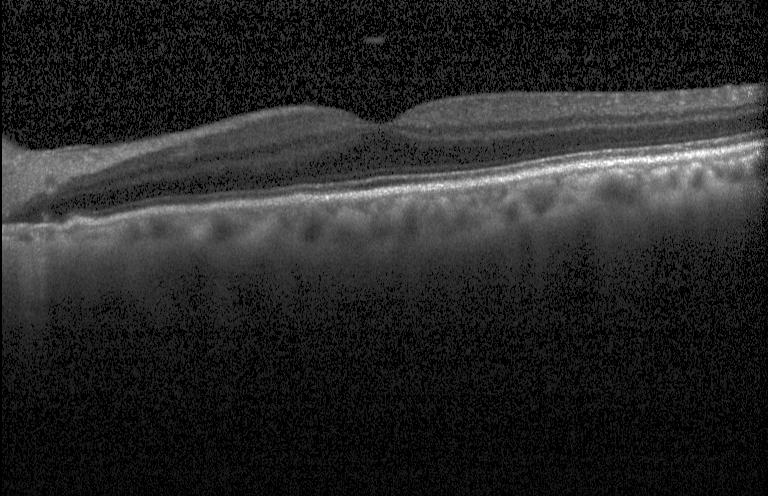

Retinal OCT B-scan — The scan shows no evidence of choroidal neovascularization, diabetic macular edema, or drusen.